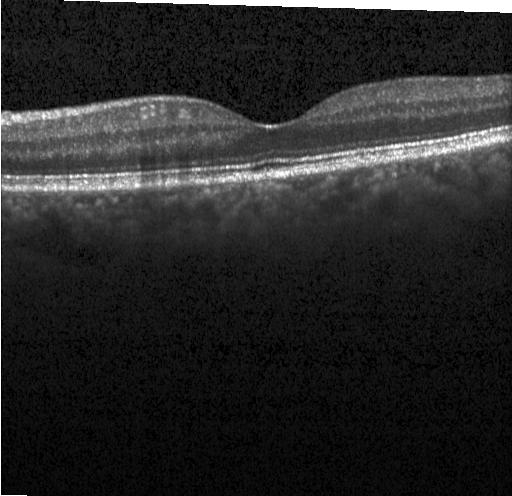

Assessment: no choroidal neovascularization, diabetic macular edema, or drusen.